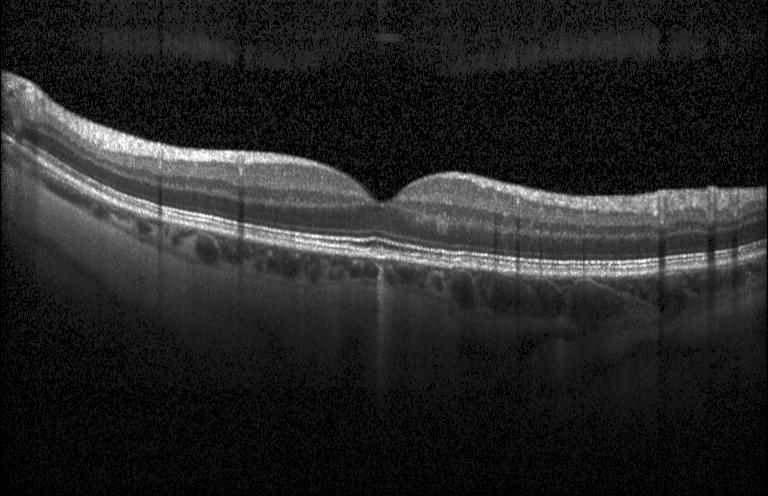
Macular OCT: neither choroidal neovascularization, diabetic macular edema, nor drusen.